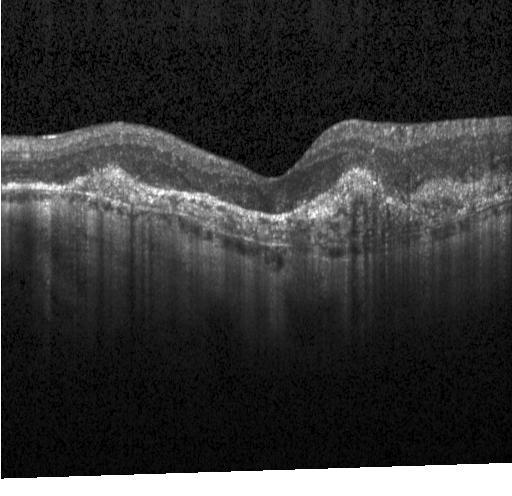

Heidelberg Spectralis OCT system; spectral-domain OCT; fovea-centered; OCT line scan — Diagnosis: choroidal neovascularization (CNV).